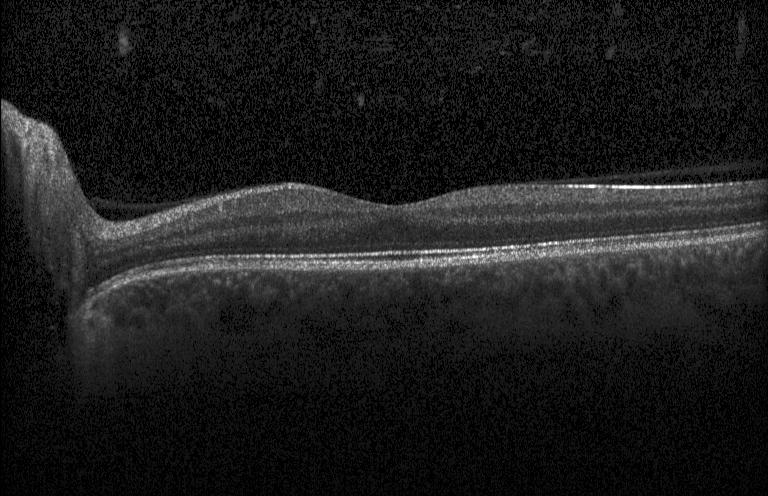 Optical coherence tomography scan, macular scan, Heidelberg Spectralis. Finding: no choroidal neovascularization, diabetic macular edema, or drusen.